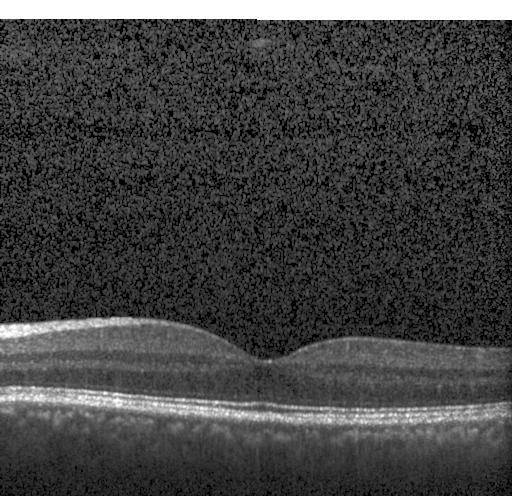 Impression: neither CNV, DME, nor drusen.